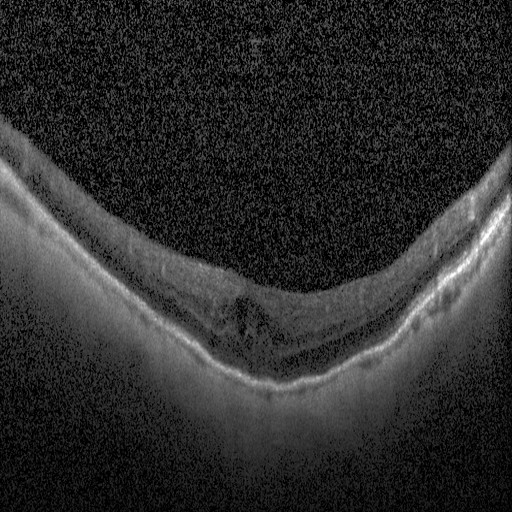

Impression: DME.